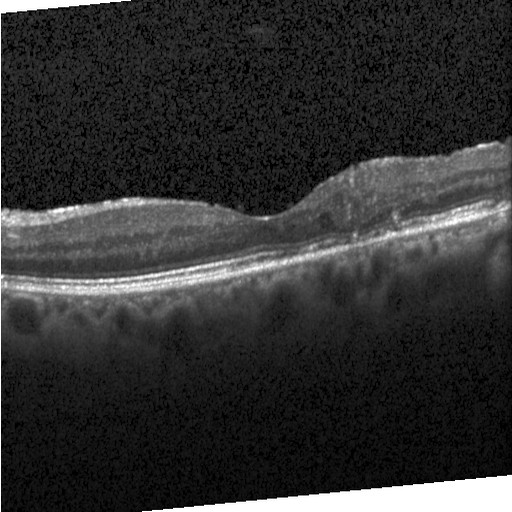

Diagnosis: diabetic macular edema.